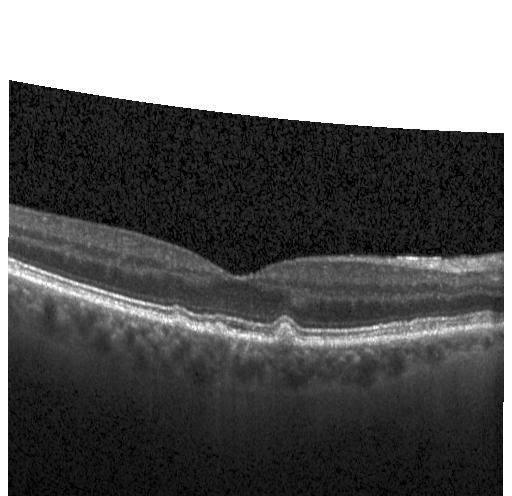
Retinal OCT cross-section.
This B-scan demonstrates multiple drusen.